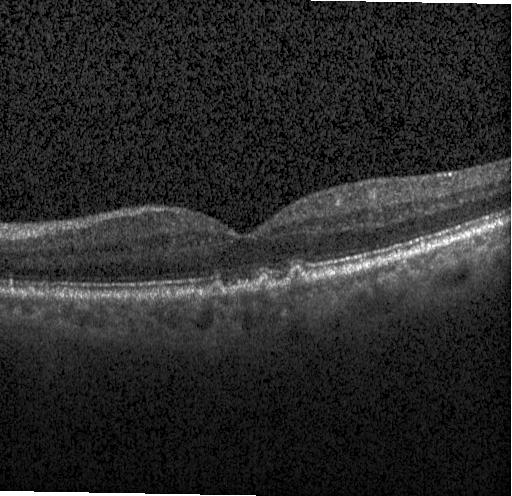 Diagnosis: drusen.